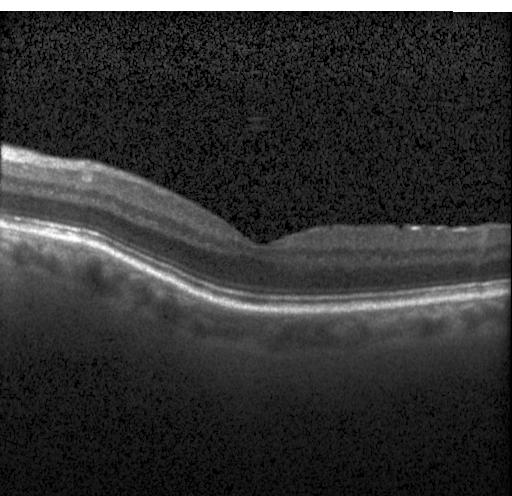

OCT line scan · Heidelberg Spectralis · macular scan · spectral-domain optical coherence tomography — Dx: no CNV, no DME, and no drusen.